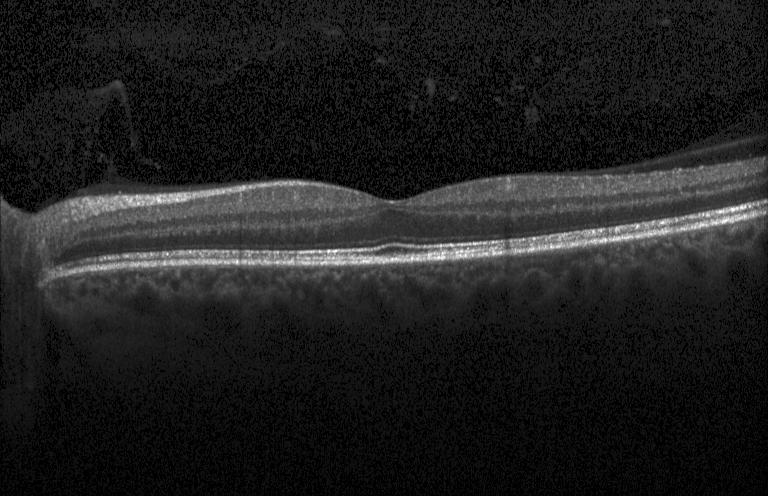
Retinal OCT B-scan; SD-OCT — Dx: no choroidal neovascularization, no diabetic macular edema, and no drusen.